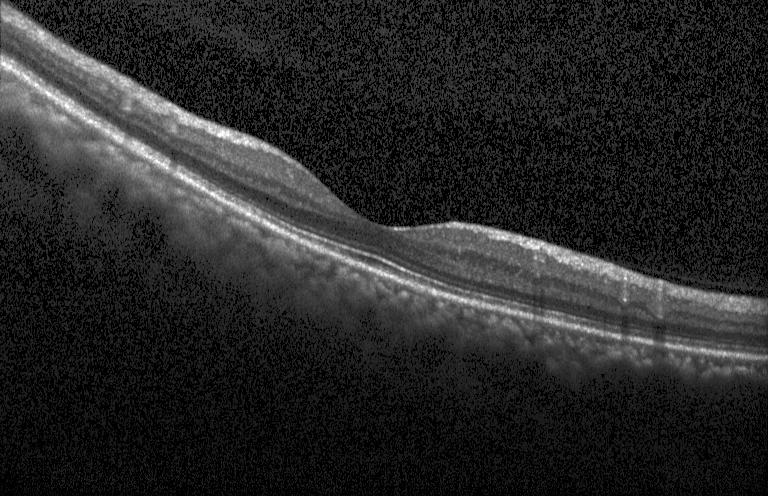 Through the macula; spectral-domain optical coherence tomography; retinal OCT B-scan; acquired on a Heidelberg Spectralis — The scan shows no choroidal neovascularization, diabetic macular edema, or drusen.